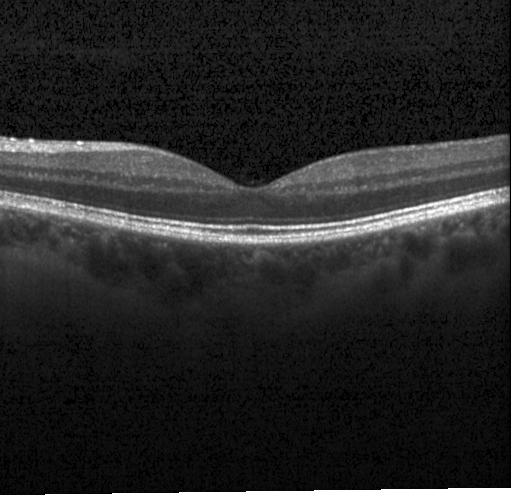

Retinal OCT cross-section; SD-OCT; horizontal scan through the fovea; acquired on a Heidelberg Spectralis
Diagnosis: no CNV, no DME, and no drusen.